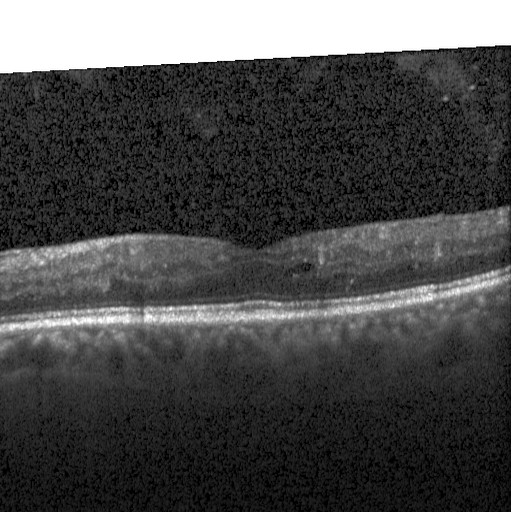
The scan shows DME.